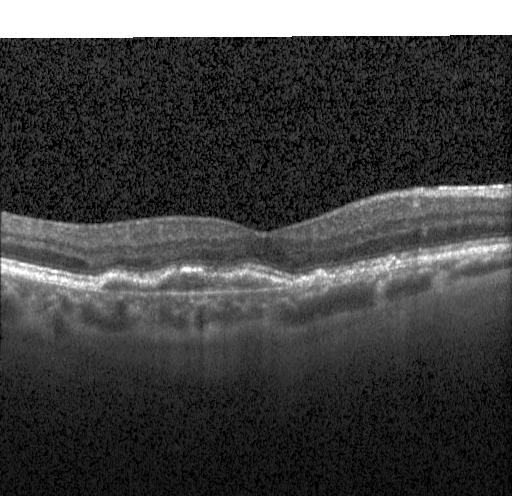
Macular OCT demonstrating a choroidal neovascular membrane.